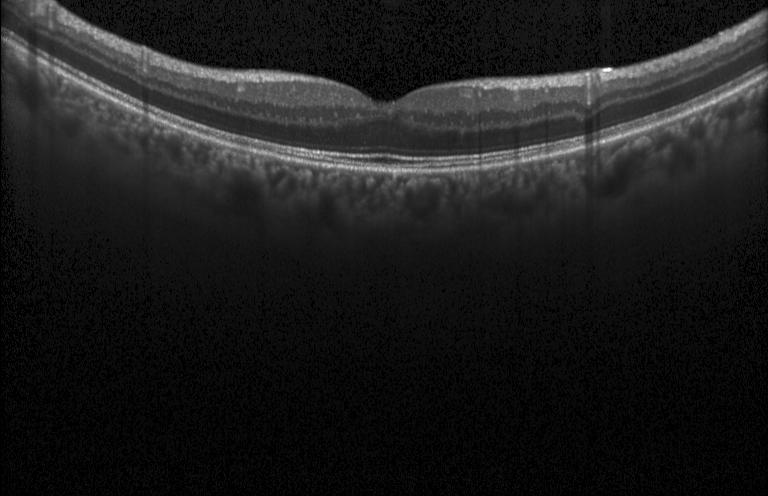
SD-OCT, OCT B-scan
Impression: no evidence of choroidal neovascularization, diabetic macular edema, or drusen.